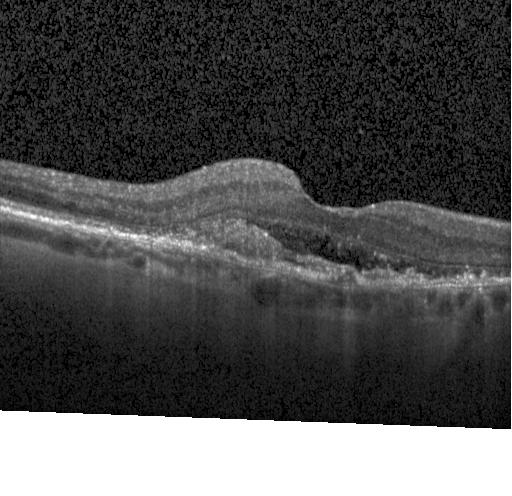 Acquired on a Heidelberg Spectralis, horizontal scan through the fovea, spectral-domain OCT, OCT line scan — Finding: choroidal neovascularization.